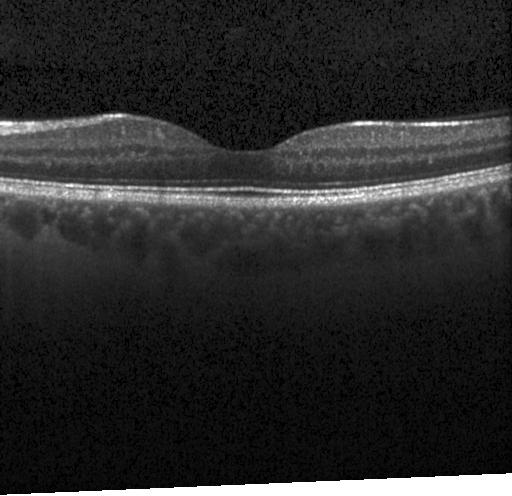
Finding: no evidence of choroidal neovascularization, diabetic macular edema, or drusen.